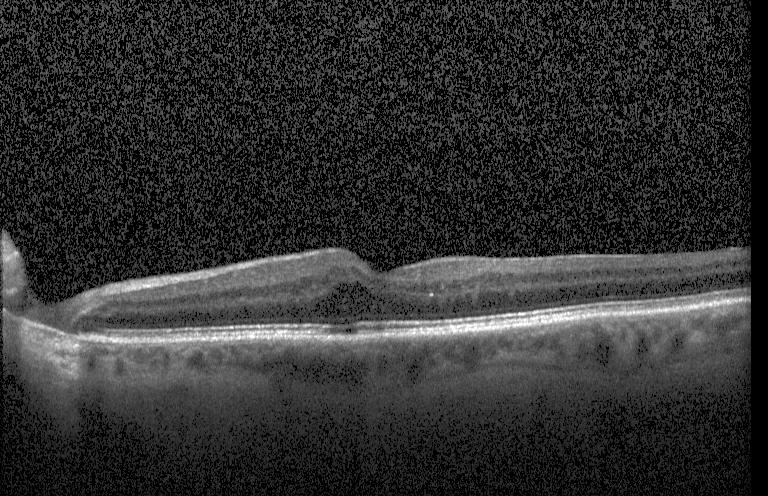 Dx: DME.